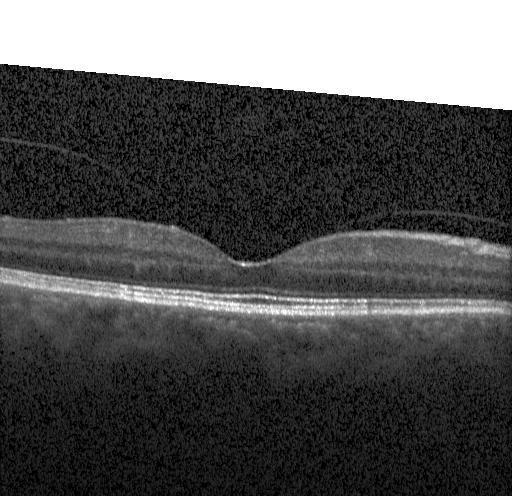
Optical coherence tomography scan, horizontal scan through the fovea, SD-OCT
This B-scan demonstrates no CNV, no DME, and no drusen.